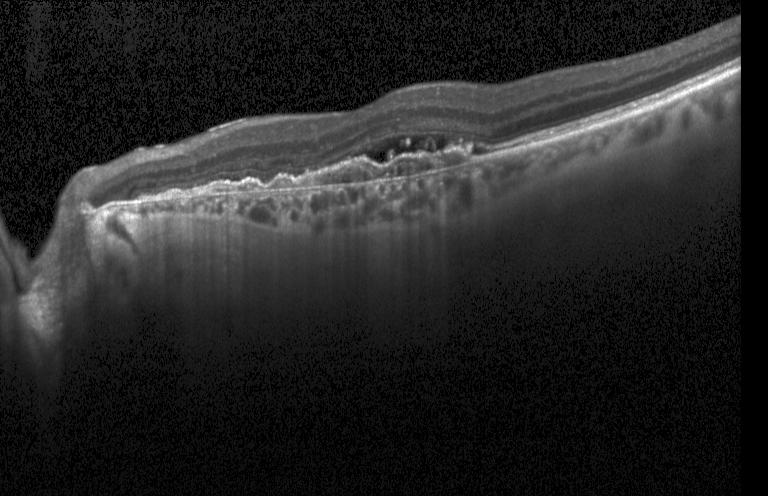

Retinal OCT cross-section.
Finding: CNV.